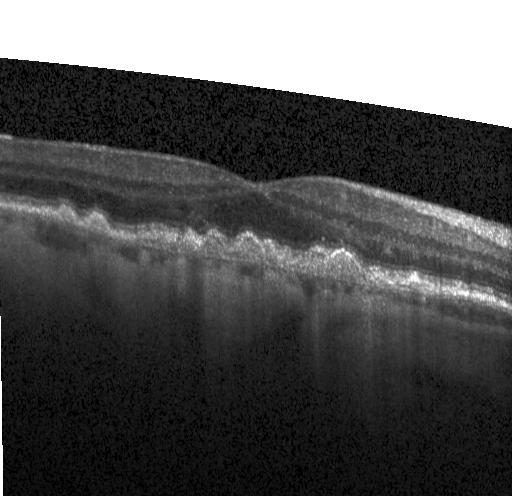
OCT B-scan — Impression: multiple drusen.